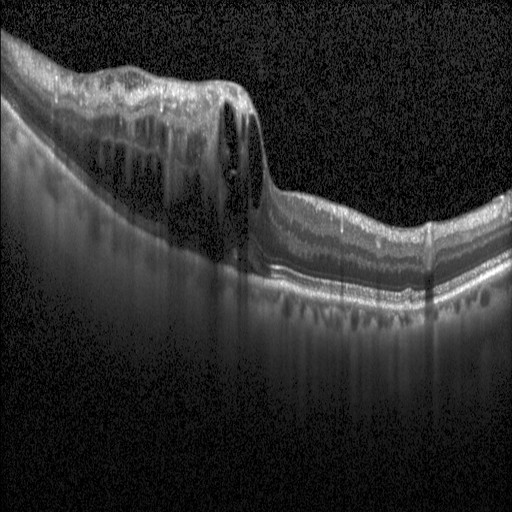

Macular OCT demonstrating diabetic macular edema.